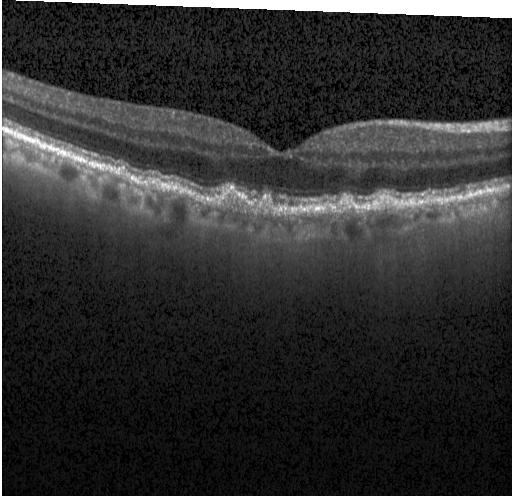 Spectral-domain optical coherence tomography. OCT B-scan
Dx: sub-RPE drusenoid deposits.